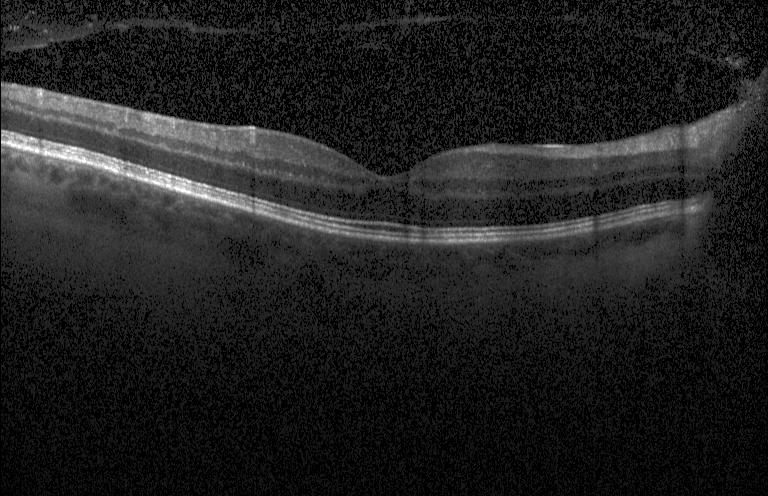 Diagnosis: neither choroidal neovascularization, diabetic macular edema, nor drusen.